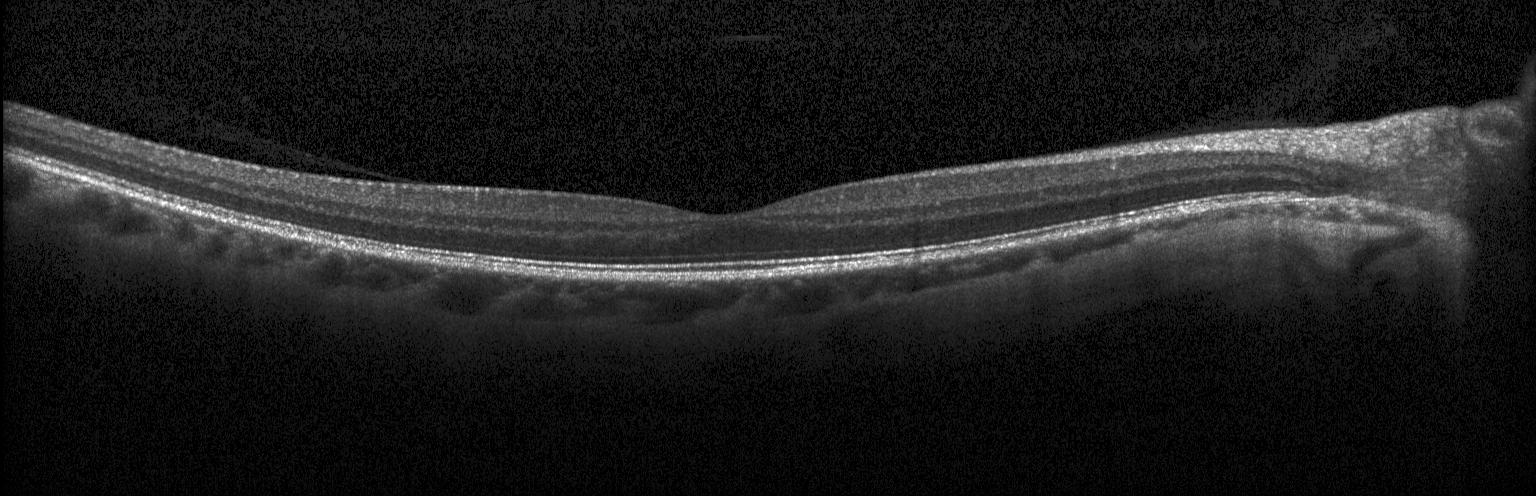 Impression: no evidence of choroidal neovascularization, diabetic macular edema, or drusen.